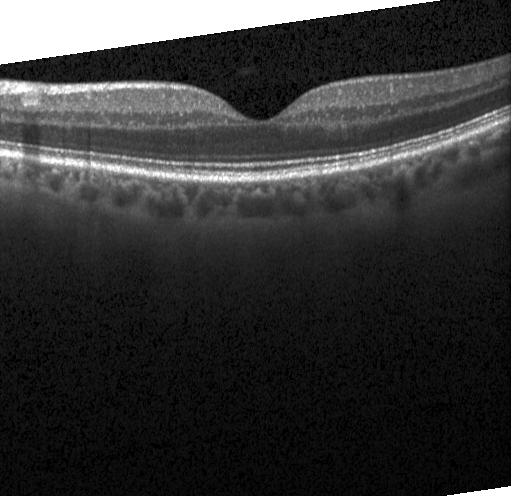 The scan shows no choroidal neovascularization, diabetic macular edema, or drusen.